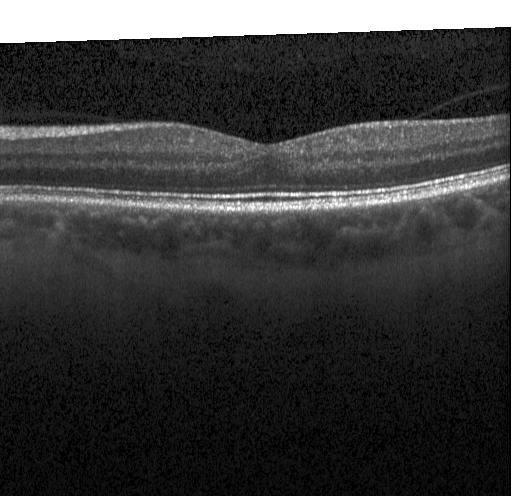 Spectral-domain optical coherence tomography · retinal OCT cross-section · fovea-centered.
The scan shows no choroidal neovascularization, diabetic macular edema, or drusen.